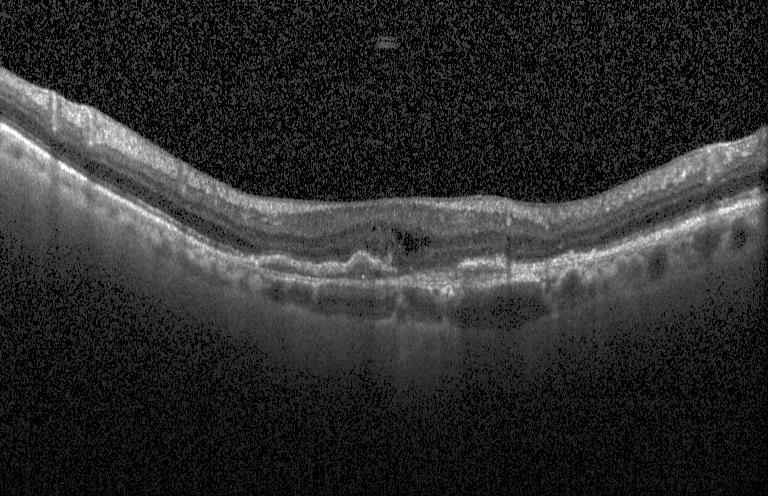 Impression: CNV.